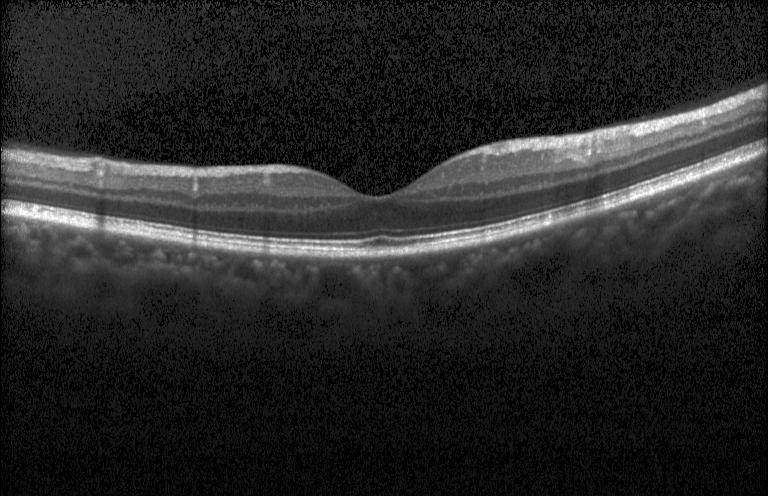
OCT B-scan; Heidelberg Spectralis; SD-OCT — Finding: no choroidal neovascularization, diabetic macular edema, or drusen.